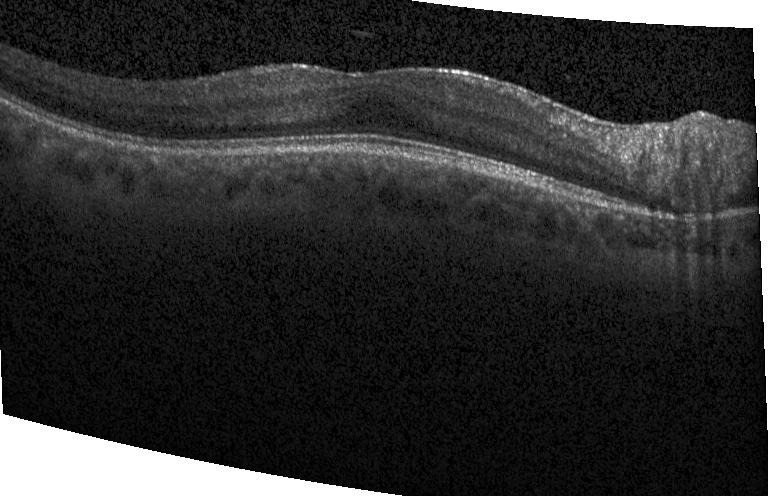
Dx: no choroidal neovascularization, diabetic macular edema, or drusen.